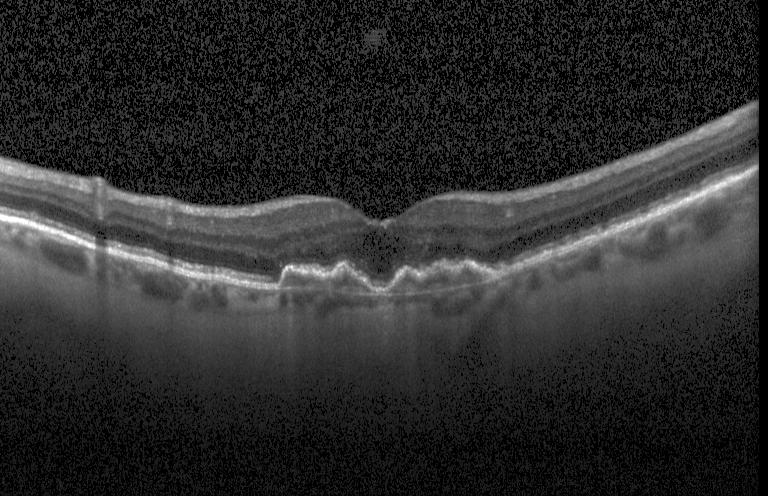

Retinal OCT cross-section.
Diagnosis: a choroidal neovascular membrane.